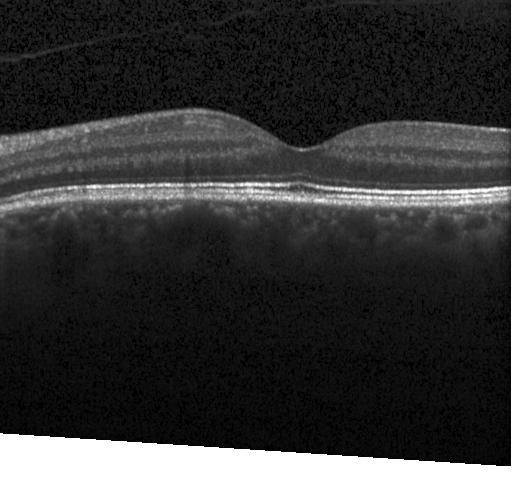

Dx: no CNV, DME, or drusen.